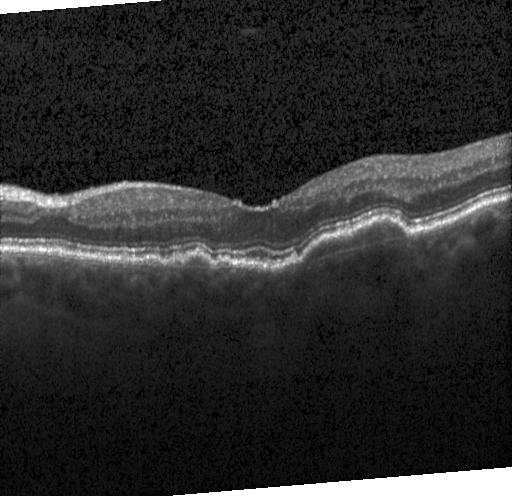

SD-OCT; through the macula; optical coherence tomography B-scan. OCT finding: a choroidal neovascular membrane.